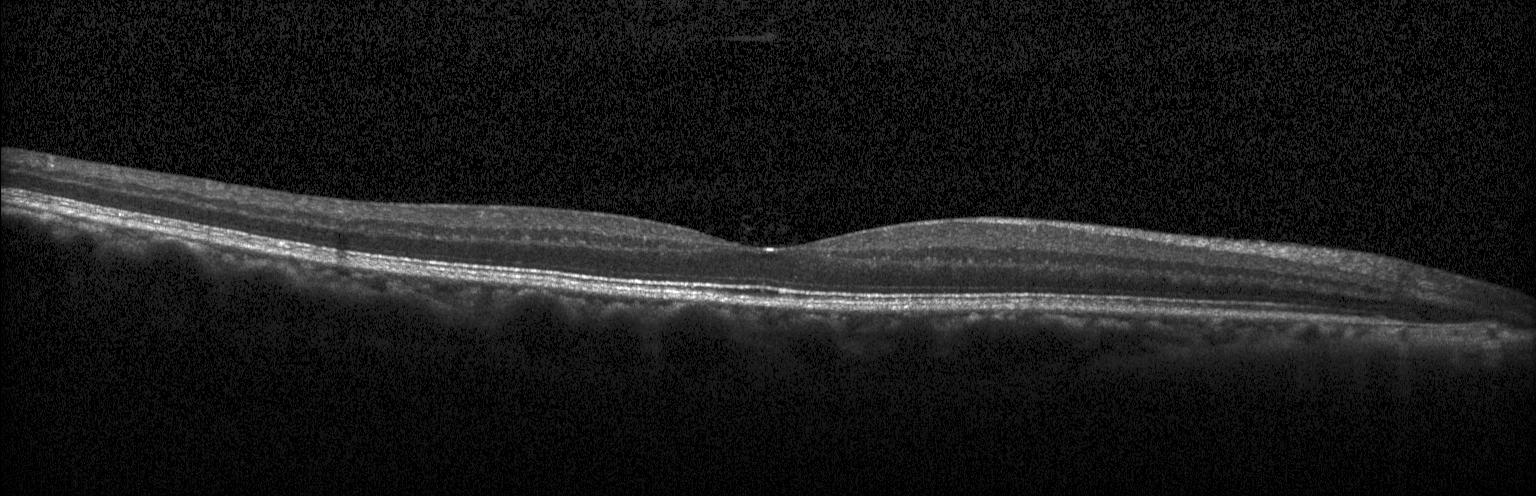
Heidelberg Spectralis OCT system; OCT line scan — The scan shows no evidence of choroidal neovascularization, diabetic macular edema, or drusen.